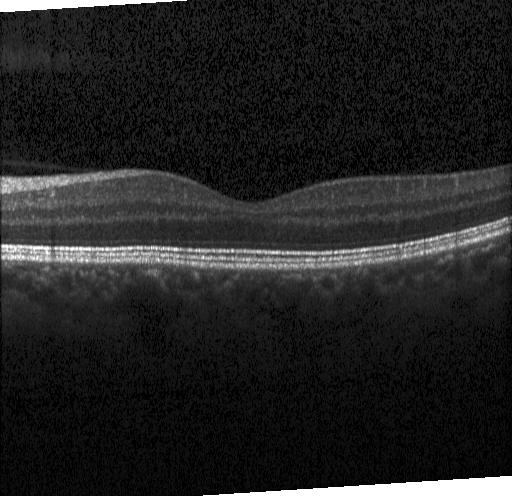

Instrument: Heidelberg Spectralis; retinal OCT B-scan; spectral-domain OCT.
The scan shows neither choroidal neovascularization, diabetic macular edema, nor drusen.